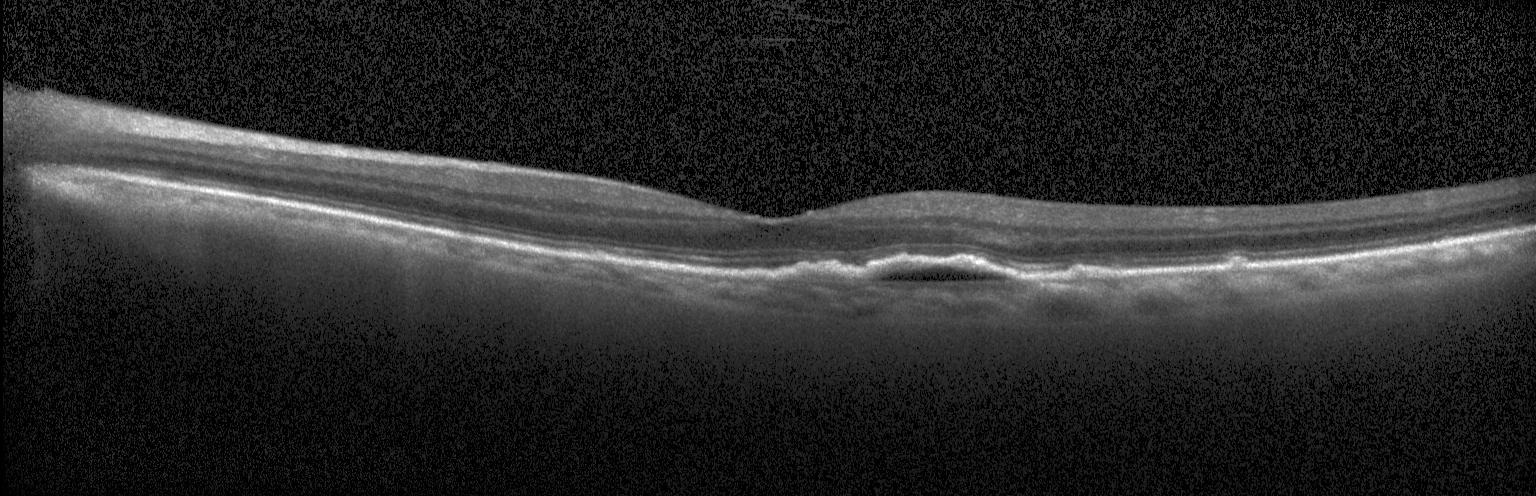
Acquired on a Heidelberg Spectralis. SD-OCT. Macular scan. Optical coherence tomography B-scan
Choroidal neovascularization.